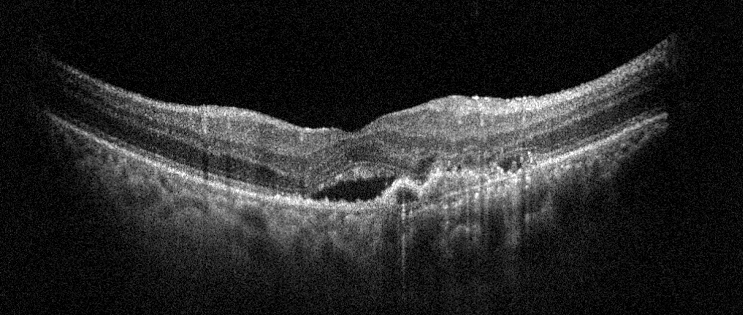 Optical coherence tomography scan. OD. This B-scan demonstrates AMD.